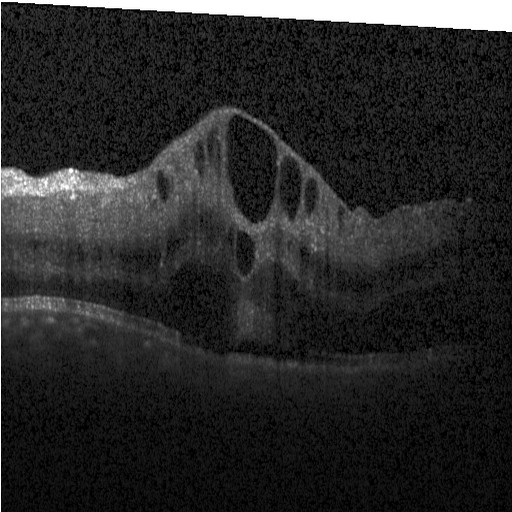 Heidelberg Spectralis. Spectral-domain OCT. Retinal OCT cross-section — Diagnosis: DME.